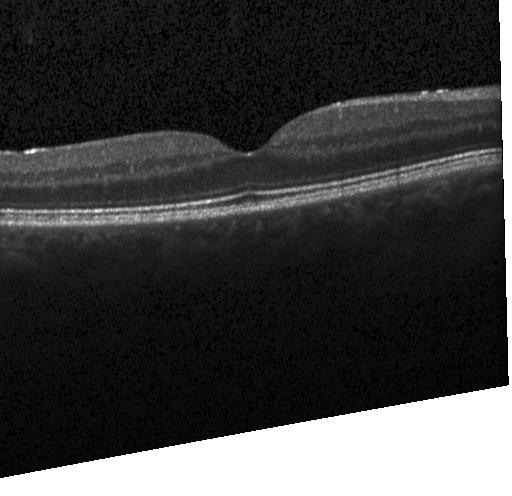
Optical coherence tomography B-scan. Finding: neither choroidal neovascularization, diabetic macular edema, nor drusen.